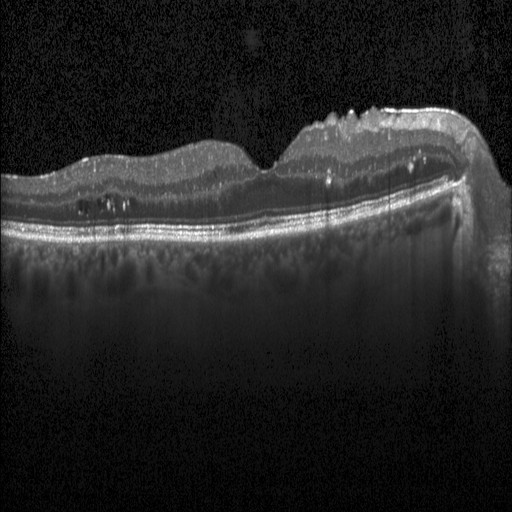 Retinal OCT cross-section.
Diagnosis: diabetic macular edema.